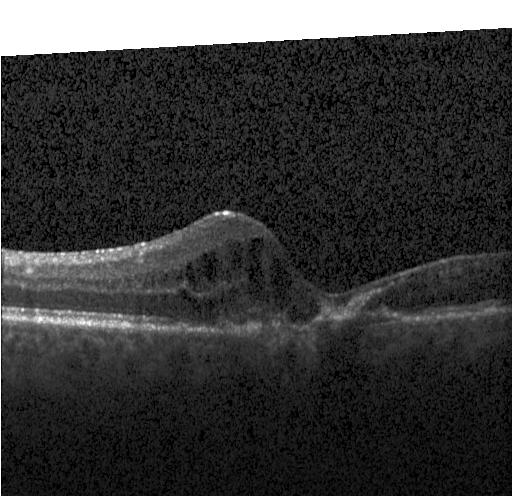 Optical coherence tomography scan.
Choroidal neovascularization (CNV).